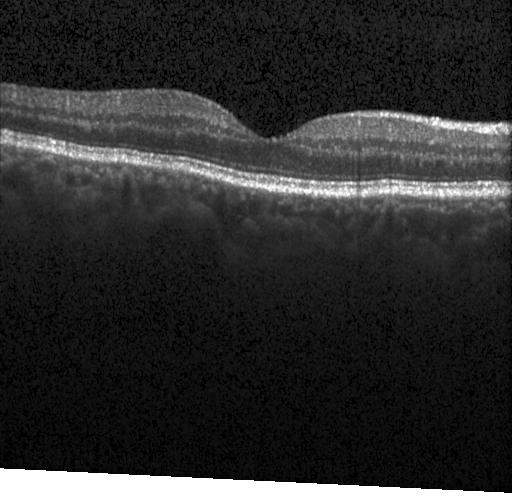

Optical coherence tomography scan · spectral-domain optical coherence tomography · macular scan · Heidelberg Spectralis — This B-scan demonstrates no CNV, no DME, and no drusen.